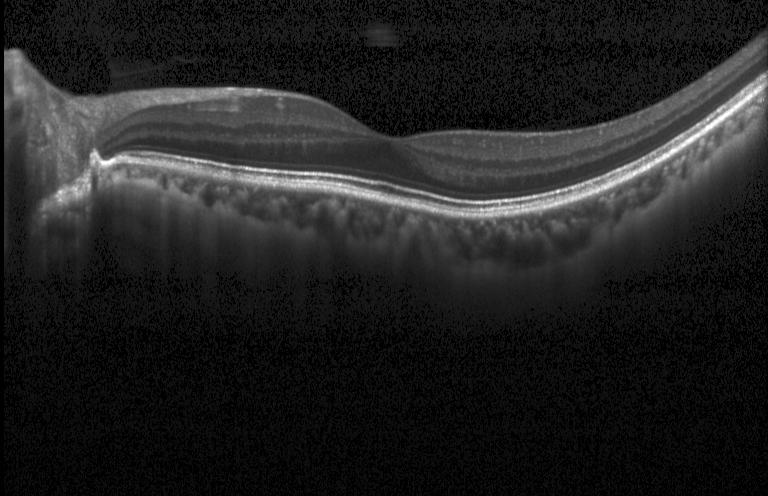 Spectral-domain OCT B-scan: no choroidal neovascularization, diabetic macular edema, or drusen.